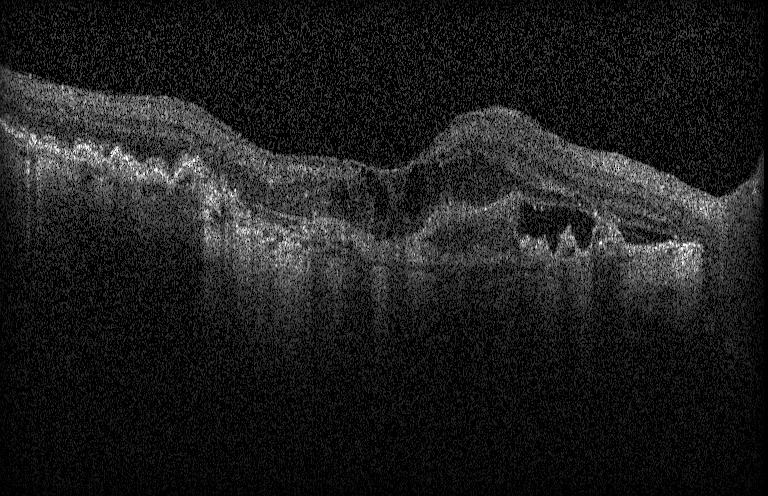 Instrument: Heidelberg Spectralis, OCT line scan, macular scan. Finding: a choroidal neovascular membrane.